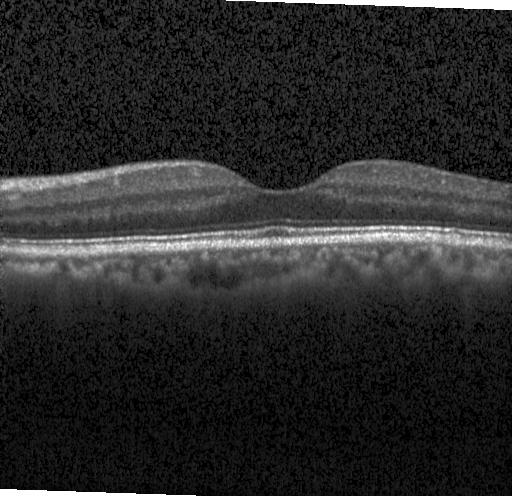
Retinal OCT cross-section showing no CNV, no DME, and no drusen.